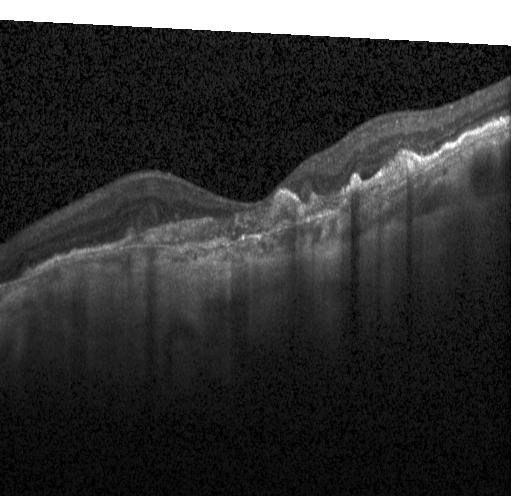
Spectral-domain optical coherence tomography. OCT line scan. Heidelberg Spectralis OCT system — Finding: a choroidal neovascular membrane.